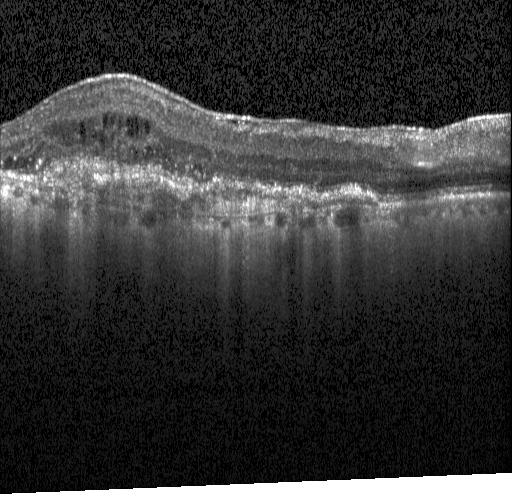

Retinal OCT cross-section showing a choroidal neovascular membrane.